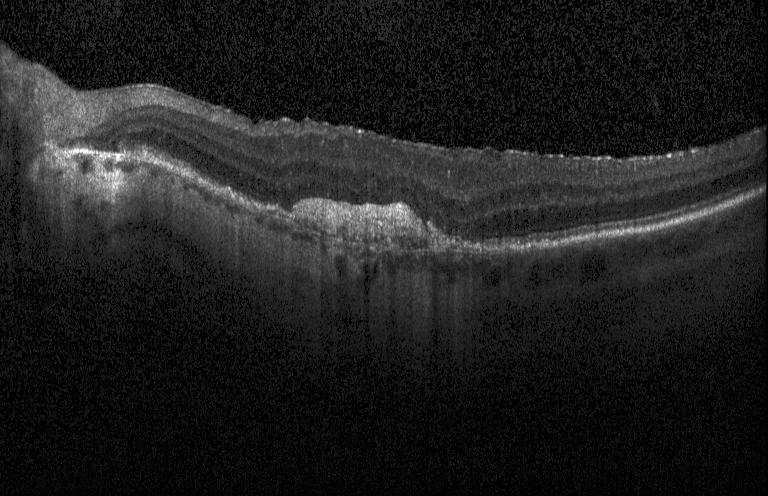

OCT line scan, horizontal scan through the fovea, spectral-domain optical coherence tomography
Macular OCT: choroidal neovascularization.